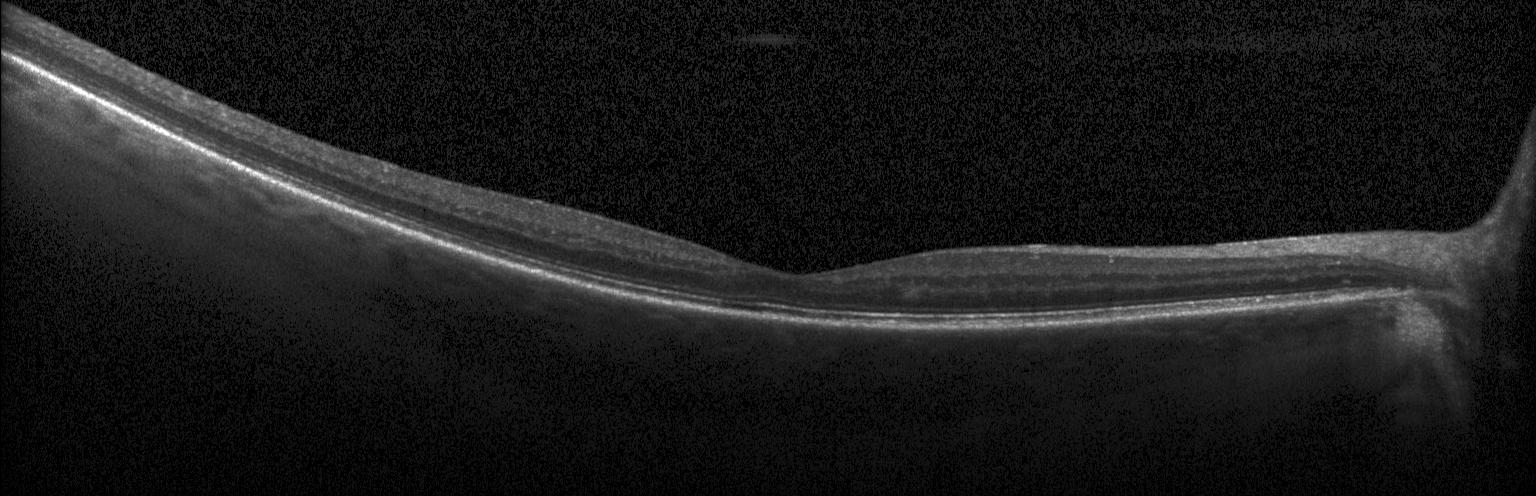

Optical coherence tomography B-scan — Assessment: no evidence of choroidal neovascularization, diabetic macular edema, or drusen.